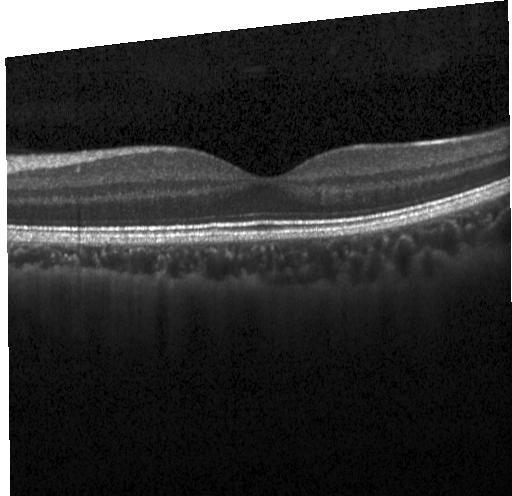 Retinal OCT cross-section — Macular OCT: no choroidal neovascularization, no diabetic macular edema, and no drusen.